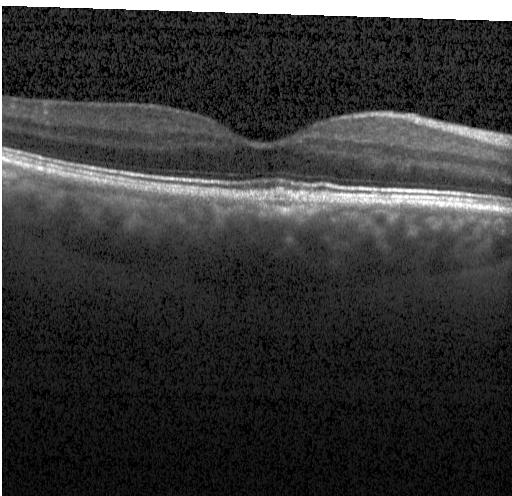

Optical coherence tomography B-scan; macular scan.
Impression: neither CNV, DME, nor drusen.